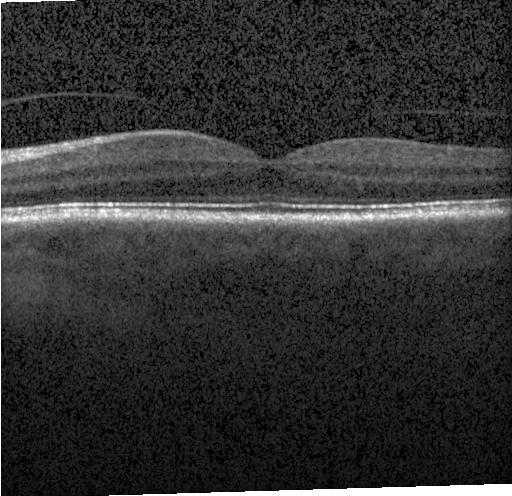
Finding: no choroidal neovascularization, diabetic macular edema, or drusen.